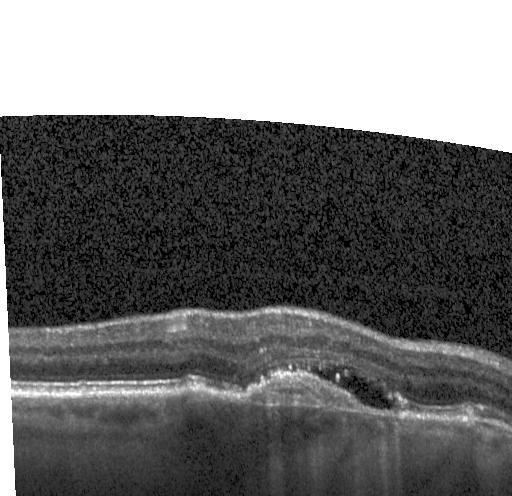
OCT line scan. OCT finding: a choroidal neovascular membrane.